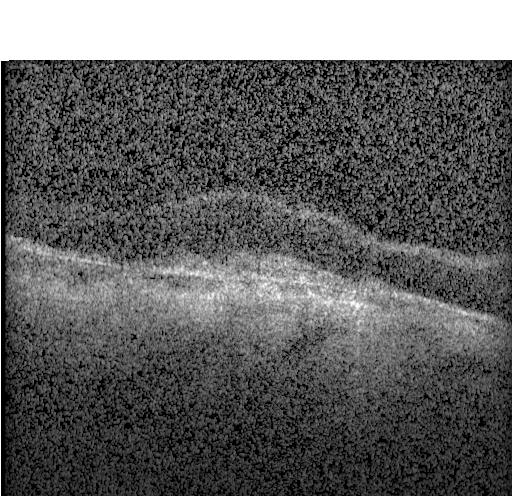 Optical coherence tomography scan · fovea-centered · SD-OCT · Heidelberg Spectralis.
This B-scan demonstrates a choroidal neovascular membrane.